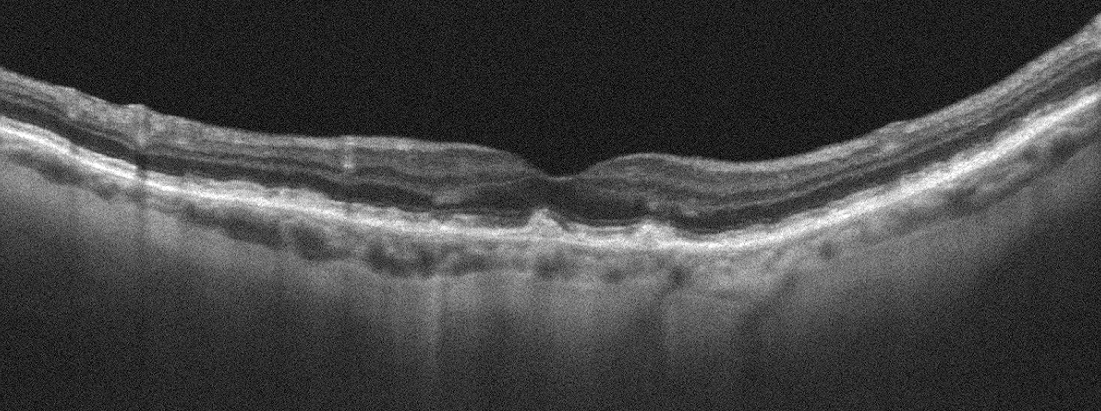

Through the macula; OCT B-scan. Finding: AMD.